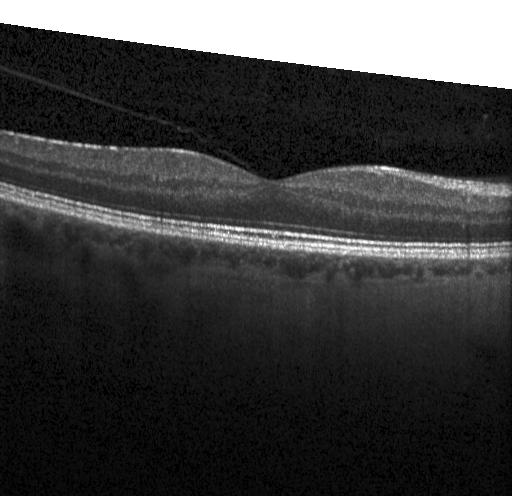

Impression: no choroidal neovascularization, diabetic macular edema, or drusen.